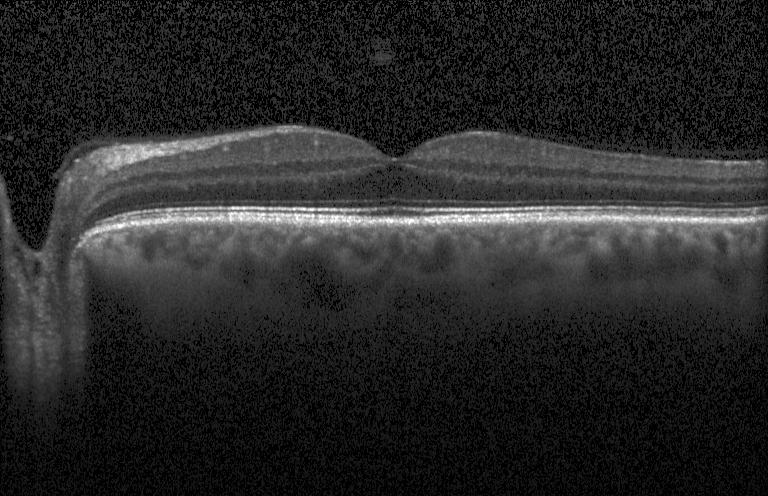 OCT B-scan showing no evidence of CNV, DME, or drusen.